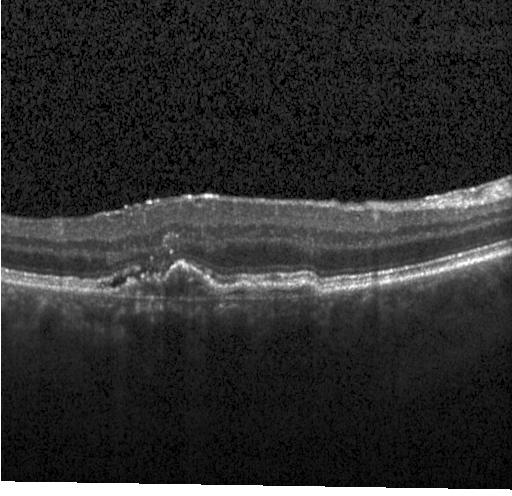 SD-OCT; through the macula; optical coherence tomography scan. Diagnosis: choroidal neovascularization (CNV).